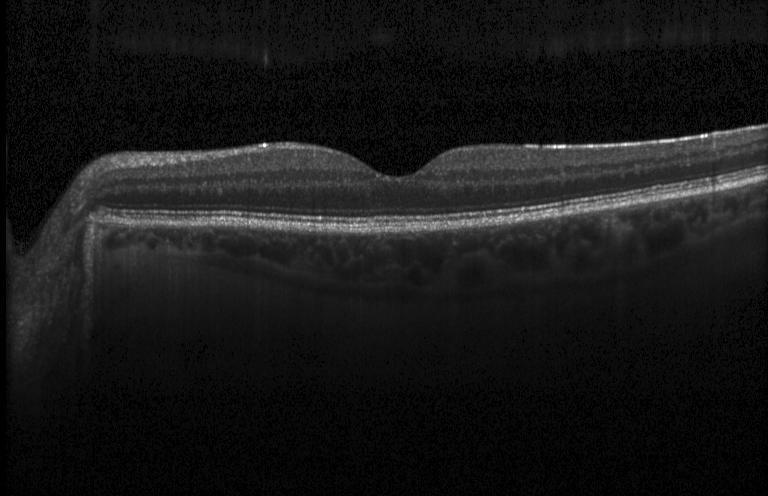

Impression: no CNV, DME, or drusen.